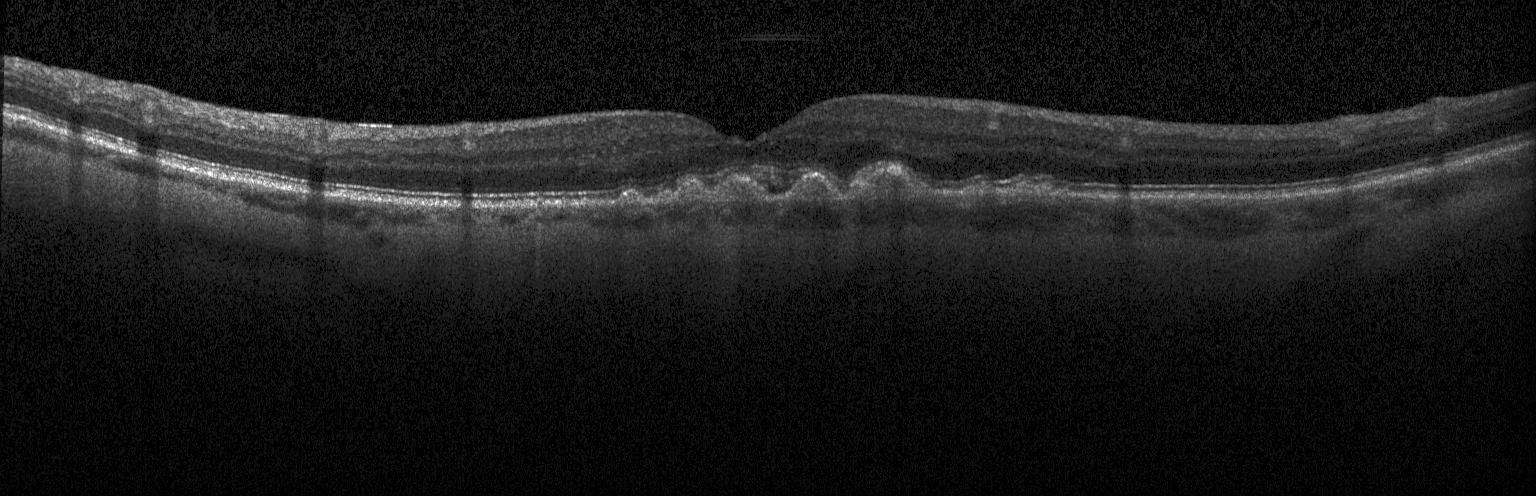 OCT line scan.
Finding: sub-RPE drusenoid deposits.